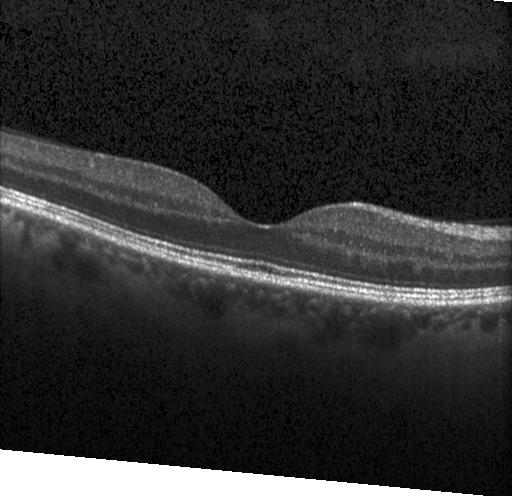
Impression: neither choroidal neovascularization, diabetic macular edema, nor drusen.